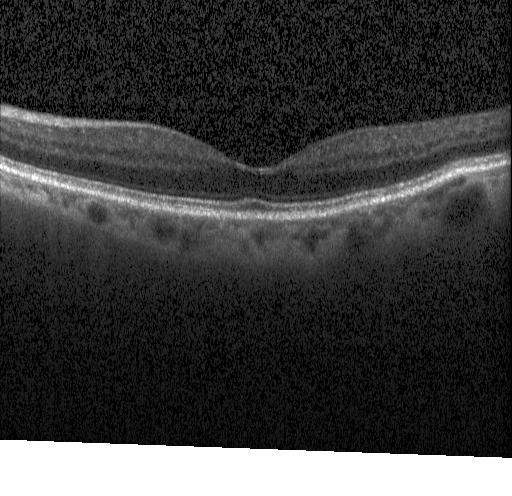
Diagnosis: neither choroidal neovascularization, diabetic macular edema, nor drusen.